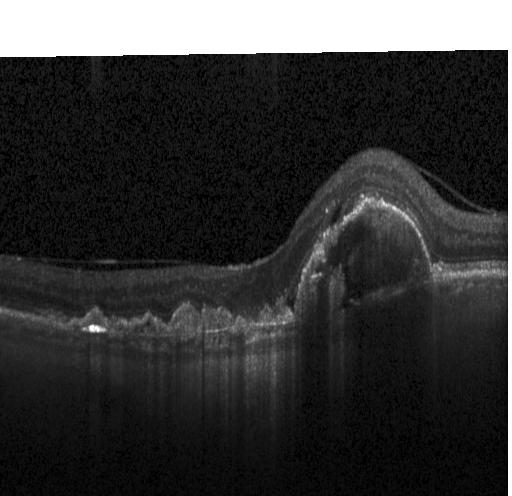
Optical coherence tomography scan. Spectral-domain OCT
A choroidal neovascular membrane.